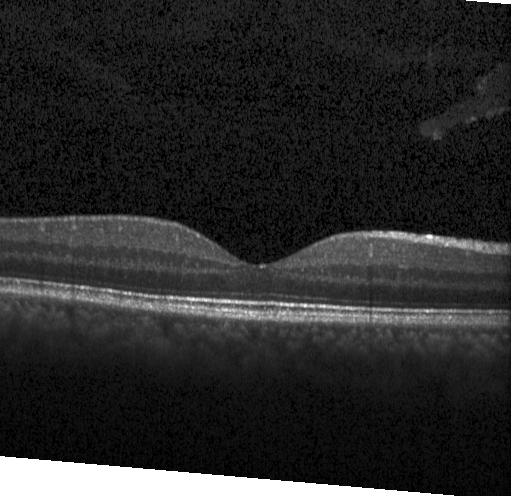 OCT B-scan, acquired on a Heidelberg Spectralis, through the macula.
This B-scan demonstrates neither choroidal neovascularization, diabetic macular edema, nor drusen.